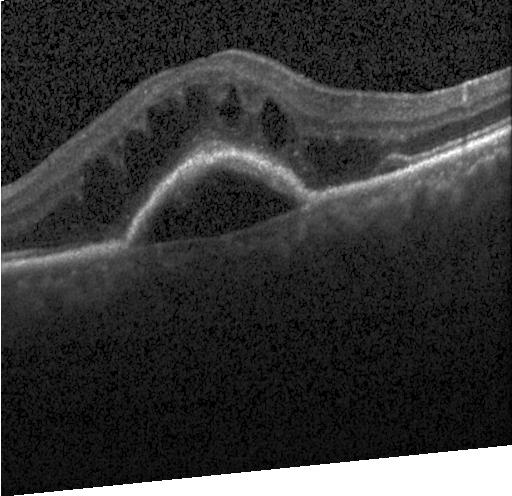 Instrument: Heidelberg Spectralis; optical coherence tomography scan; through the macula; SD-OCT. Finding: a choroidal neovascular membrane.